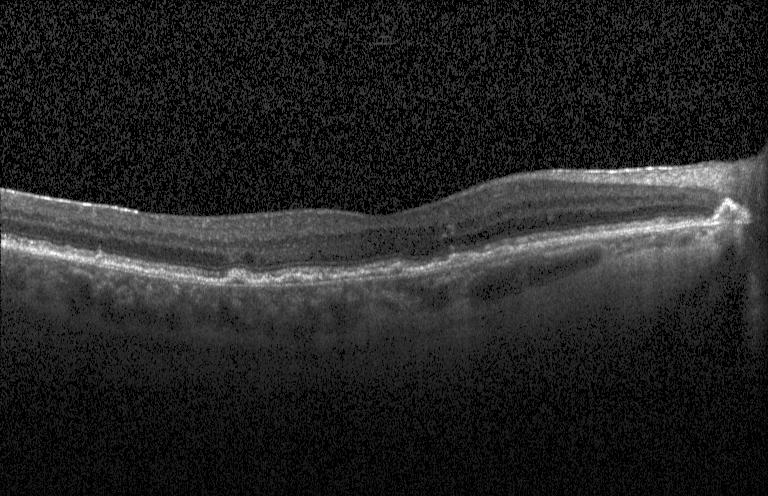
Retinal OCT B-scan
Impression: CNV.